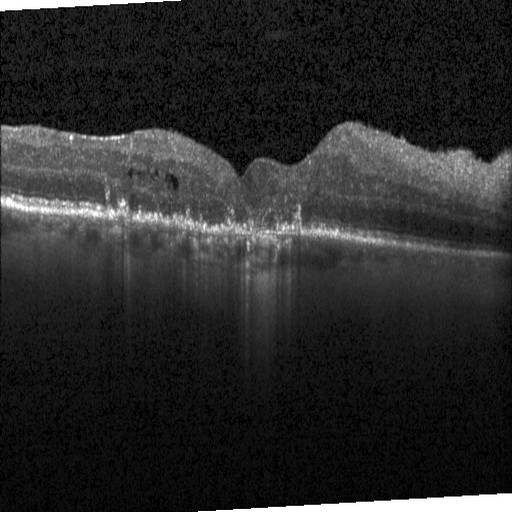
Retinal OCT cross-section
OCT finding: diabetic macular edema (DME).